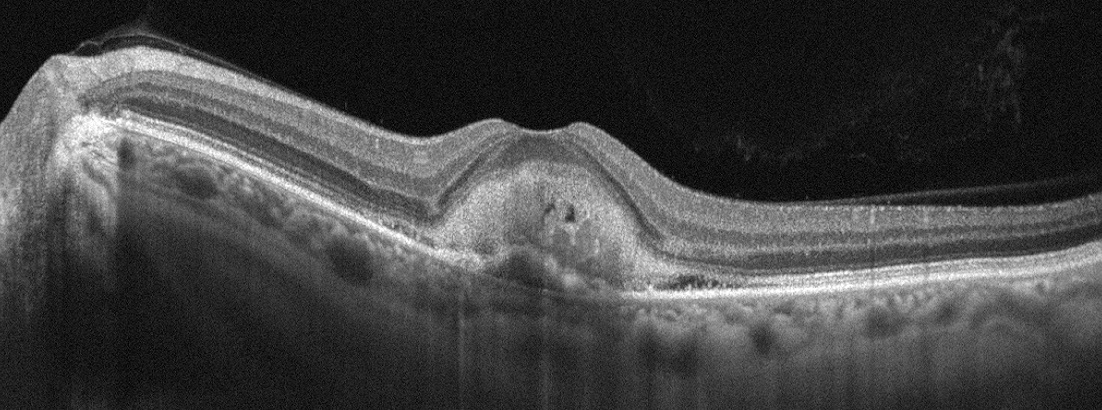

Optical coherence tomography B-scan. The scan shows age-related macular degeneration (AMD).